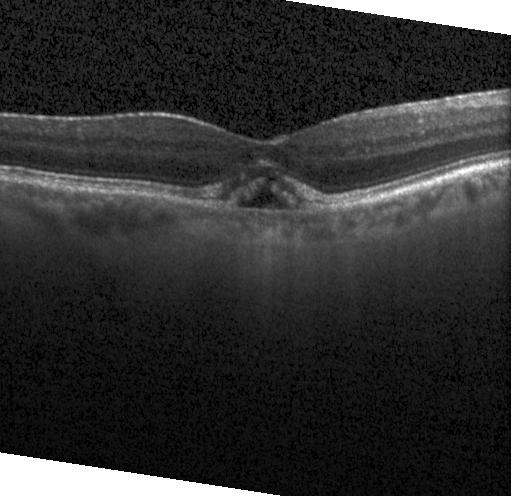
Spectral-domain OCT, retinal OCT cross-section, through the macula. Finding: choroidal neovascularization.